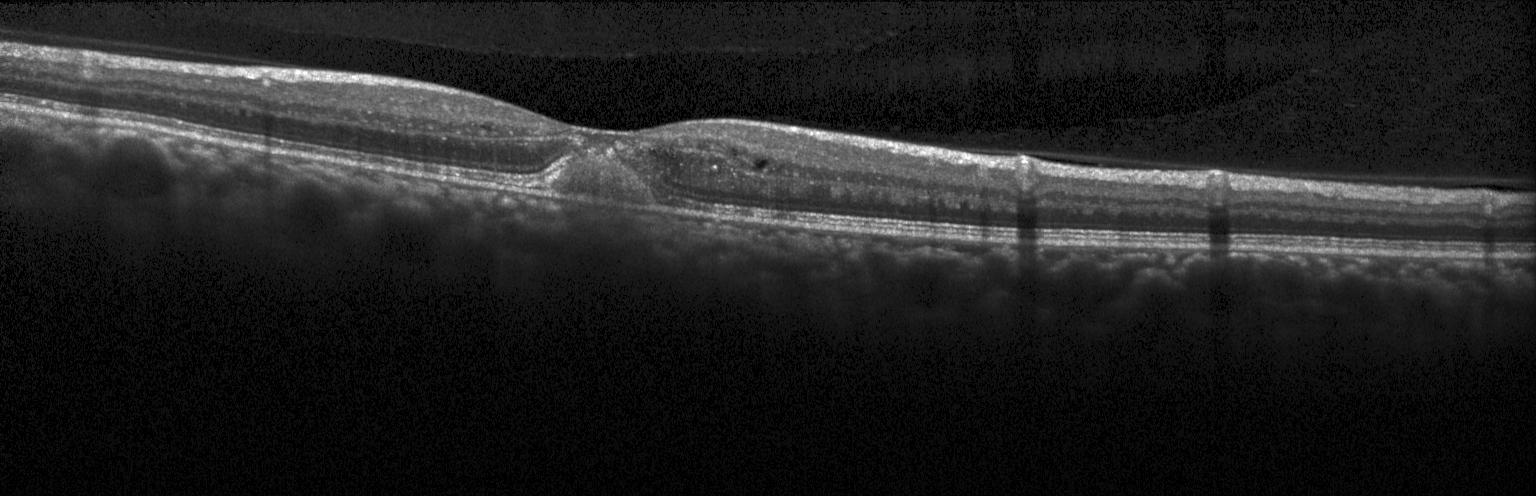
Retinal OCT B-scan · Heidelberg Spectralis OCT system · spectral-domain OCT · fovea-centered. Diagnosis: a choroidal neovascular membrane.